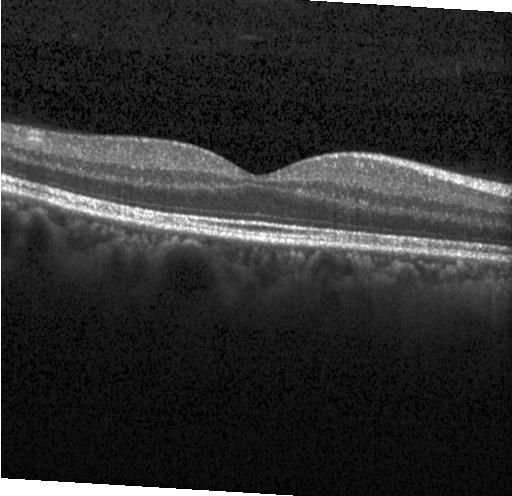 Centered on the fovea · OCT line scan · acquired on a Heidelberg Spectralis · spectral-domain optical coherence tomography — Finding: no CNV, no DME, and no drusen.